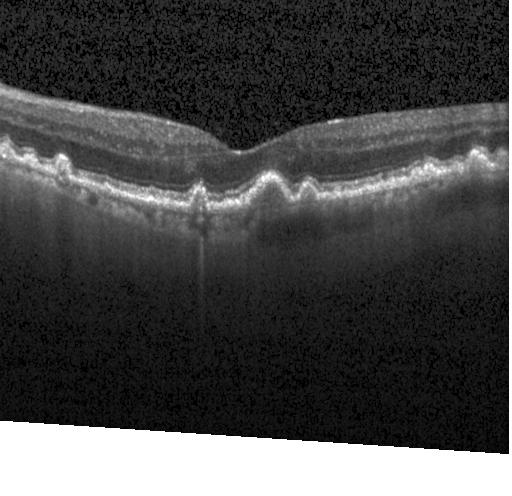
Instrument: Heidelberg Spectralis; optical coherence tomography scan — Diagnosis: drusen.